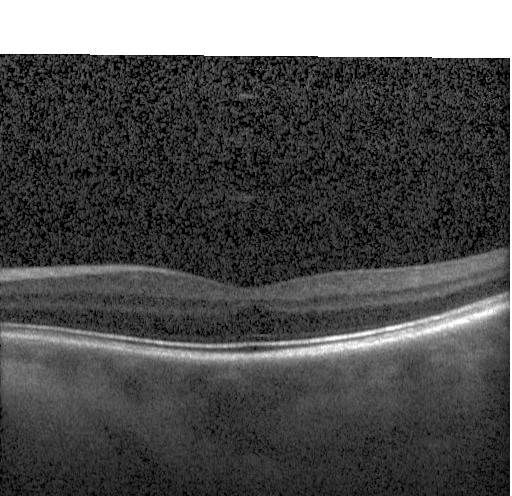

Macular scan. Retinal OCT B-scan. Spectral-domain optical coherence tomography. Heidelberg Spectralis — Finding: no evidence of choroidal neovascularization, diabetic macular edema, or drusen.